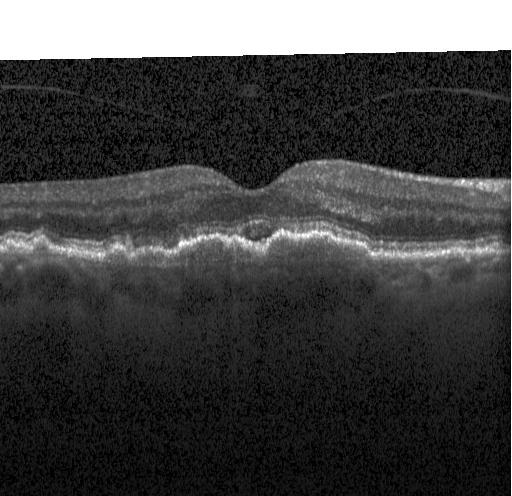 Optical coherence tomography B-scan · SD-OCT · through the macula · Heidelberg Spectralis — Macular OCT: a choroidal neovascular membrane.